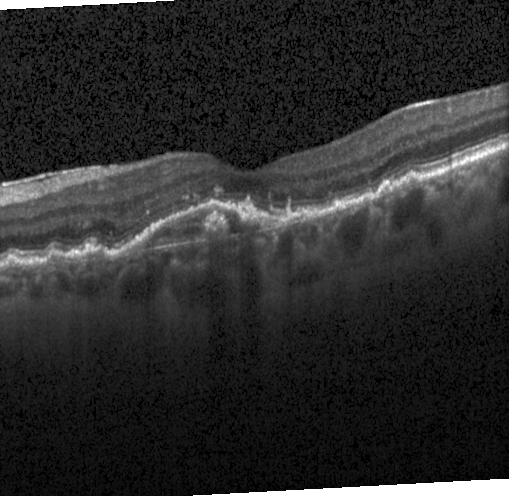

Optical coherence tomography scan · instrument: Heidelberg Spectralis · horizontal scan through the fovea · SD-OCT. The scan shows a choroidal neovascular membrane.